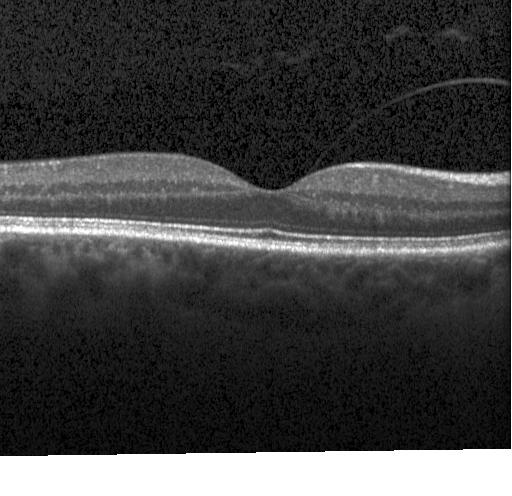
Dx: neither choroidal neovascularization, diabetic macular edema, nor drusen.